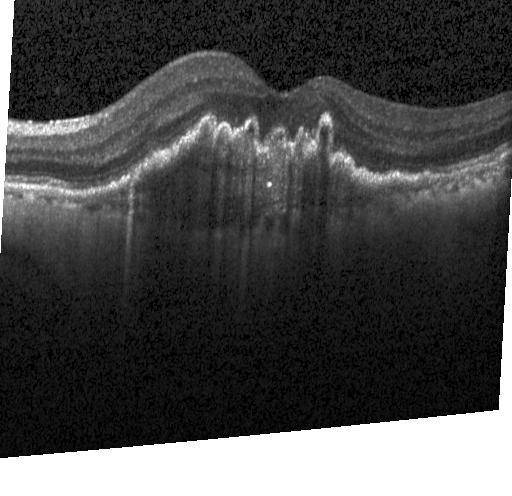

OCT line scan — Diagnosis: a choroidal neovascular membrane.